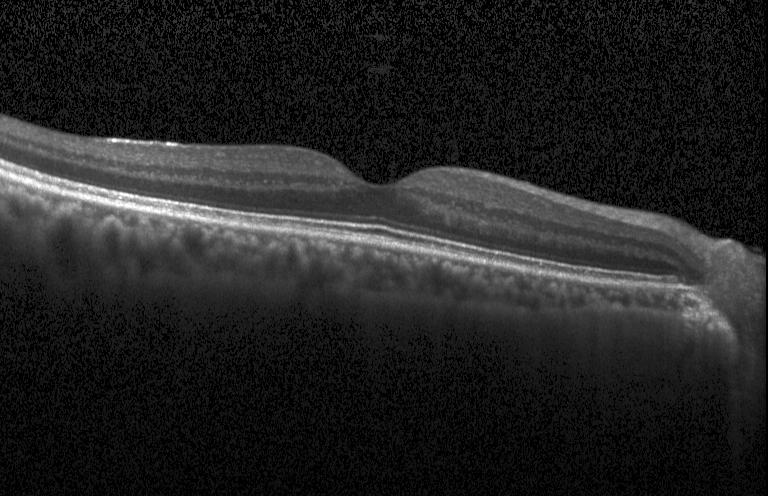
Finding: no evidence of choroidal neovascularization, diabetic macular edema, or drusen.